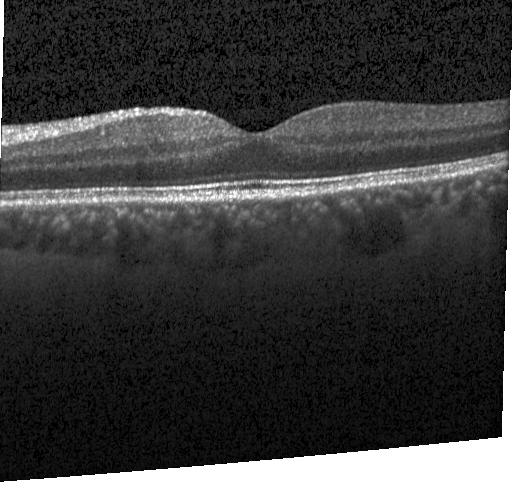
Optical coherence tomography B-scan. Horizontal scan through the fovea
Impression: no choroidal neovascularization, diabetic macular edema, or drusen.